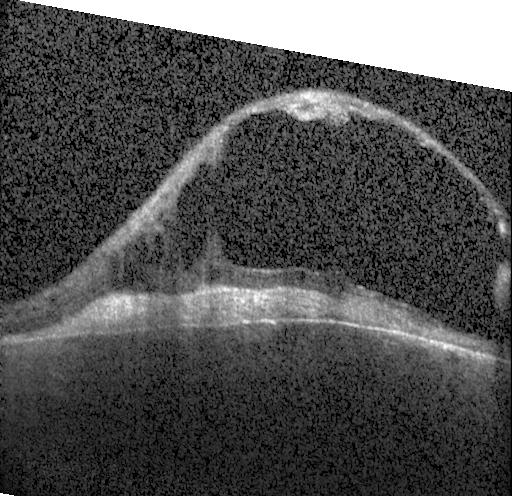
Spectral-domain OCT · OCT B-scan — The scan shows a choroidal neovascular membrane.